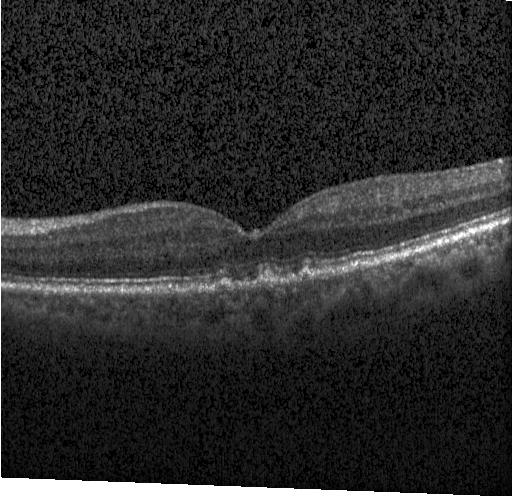
Spectral-domain OCT; OCT B-scan. Impression: multiple drusen.